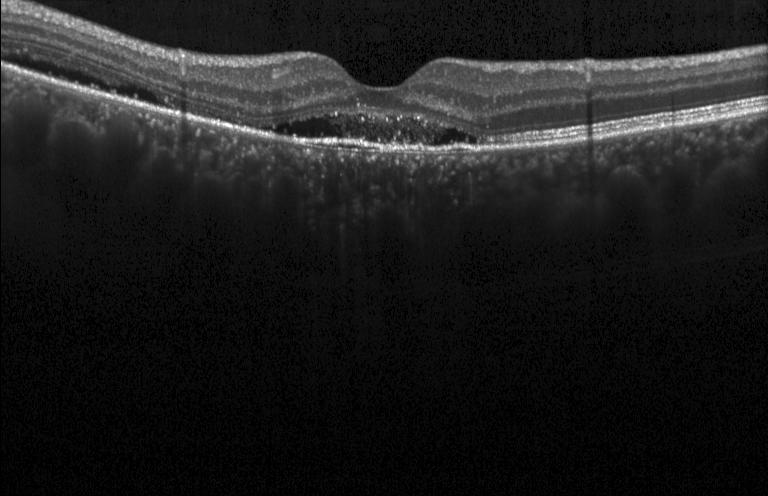 Optical coherence tomography B-scan
The scan shows a choroidal neovascular membrane.